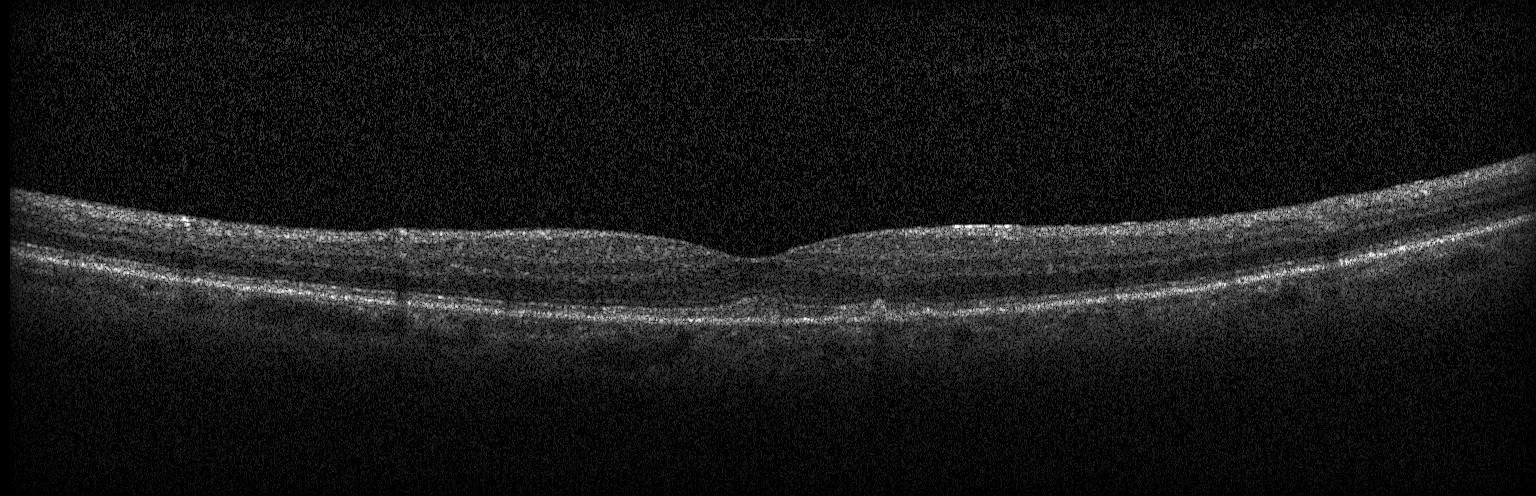 Assessment: multiple drusen.